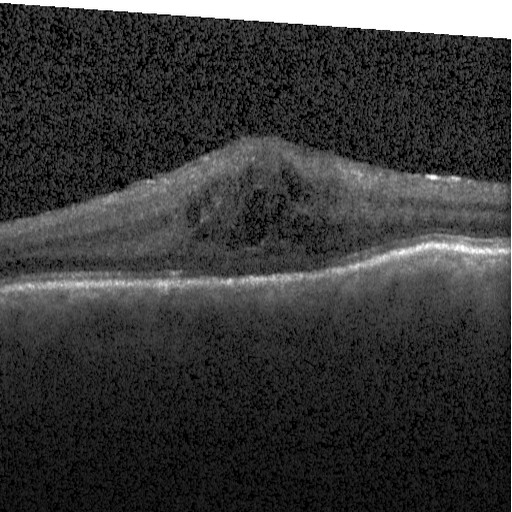
Acquired on a Heidelberg Spectralis · optical coherence tomography B-scan — The scan shows diabetic macular edema.